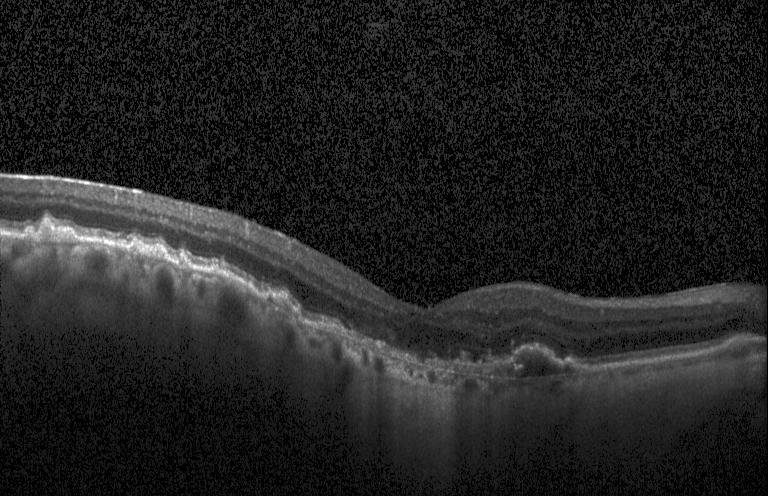 Instrument: Heidelberg Spectralis, retinal OCT B-scan — Finding: choroidal neovascularization (CNV).